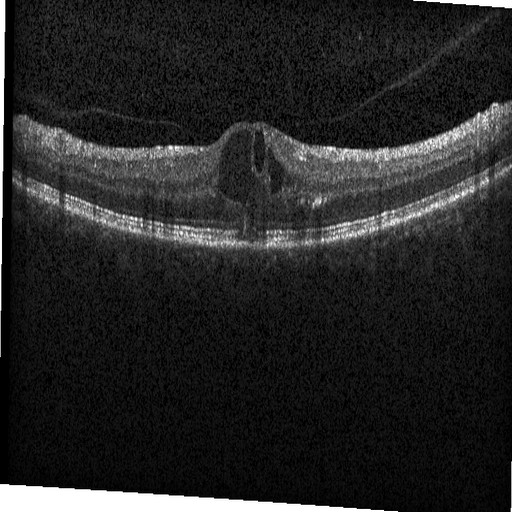

Acquired on a Heidelberg Spectralis; retinal OCT B-scan; spectral-domain optical coherence tomography; through the macula — OCT finding: diabetic macular edema.